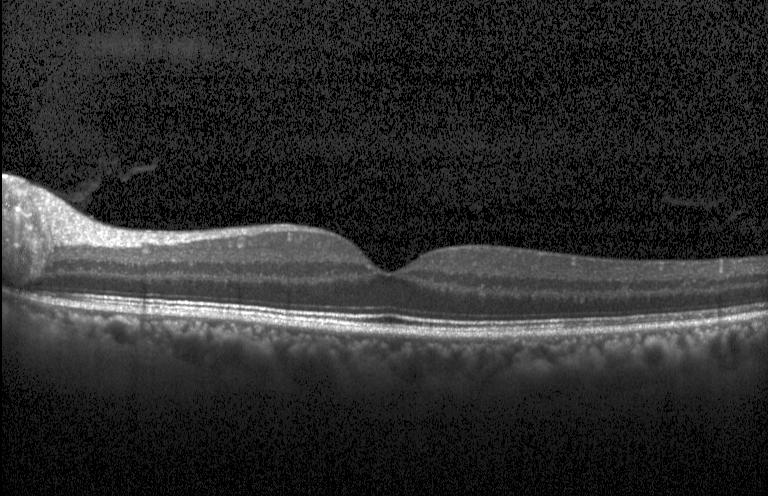

Spectral-domain optical coherence tomography · horizontal scan through the fovea · optical coherence tomography scan. Finding: no evidence of choroidal neovascularization, diabetic macular edema, or drusen.